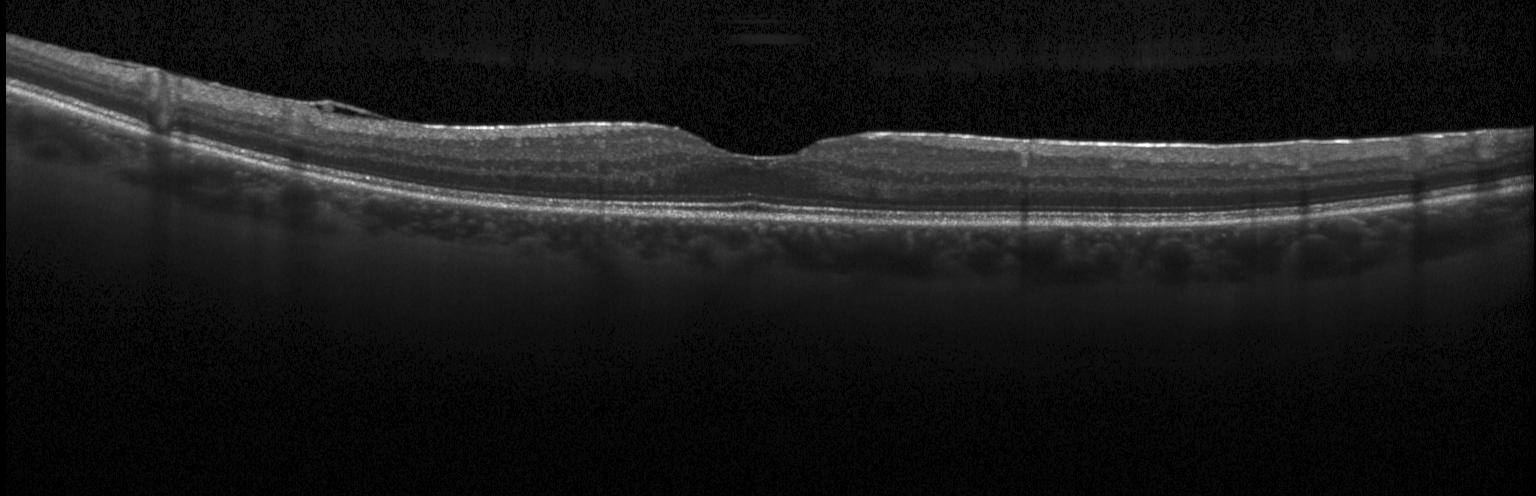 Diagnosis: neither choroidal neovascularization, diabetic macular edema, nor drusen.